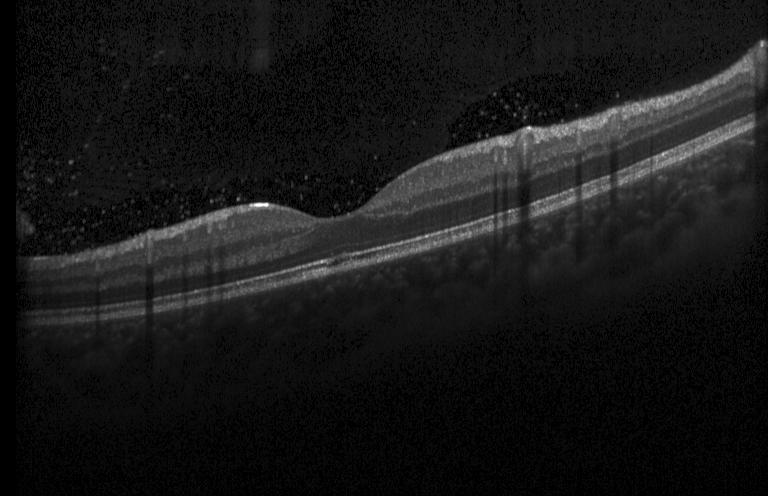 Macular scan; OCT B-scan
Impression: no evidence of CNV, DME, or drusen.